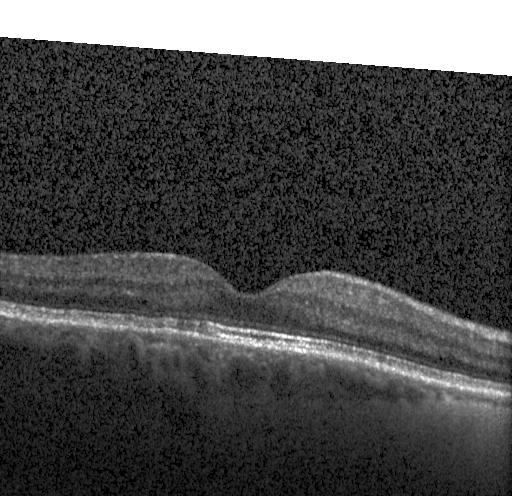

Optical coherence tomography scan.
Assessment: no evidence of choroidal neovascularization, diabetic macular edema, or drusen.